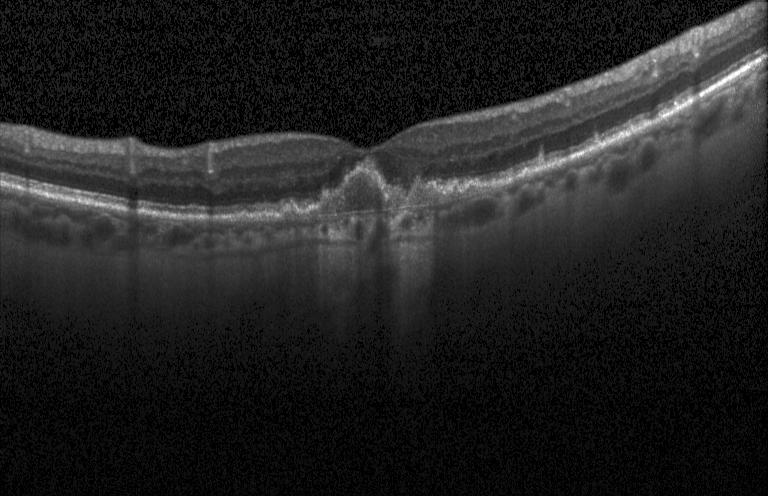
Retinal OCT B-scan — Dx: CNV.